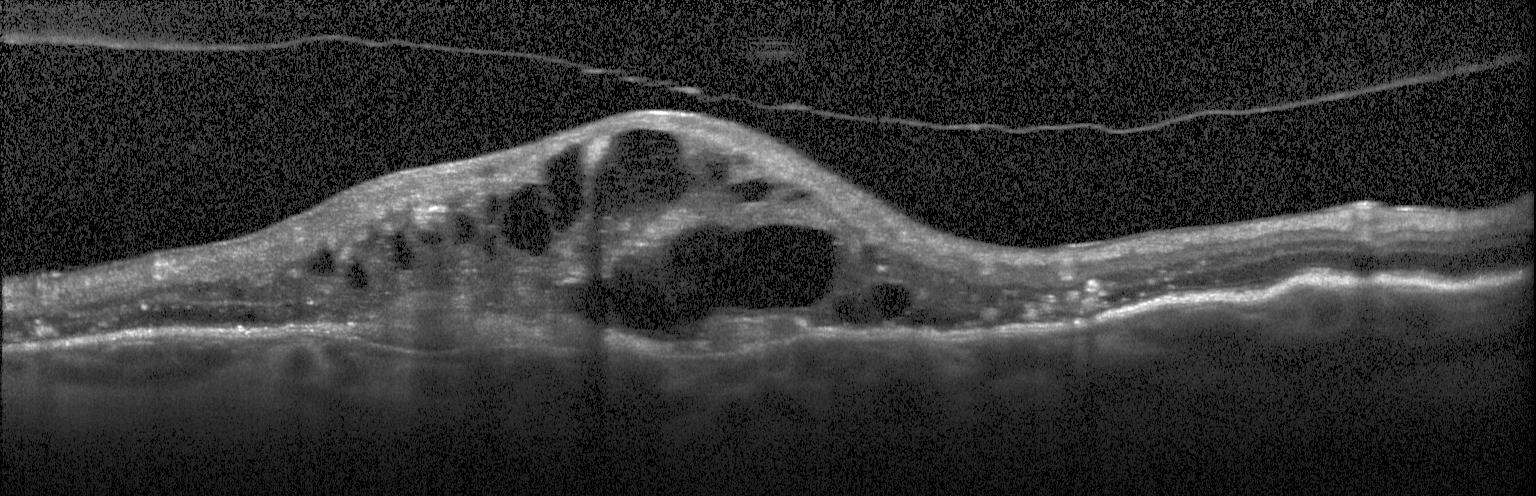
Spectral-domain optical coherence tomography, fovea-centered, retinal OCT cross-section — OCT finding: choroidal neovascularization (CNV).